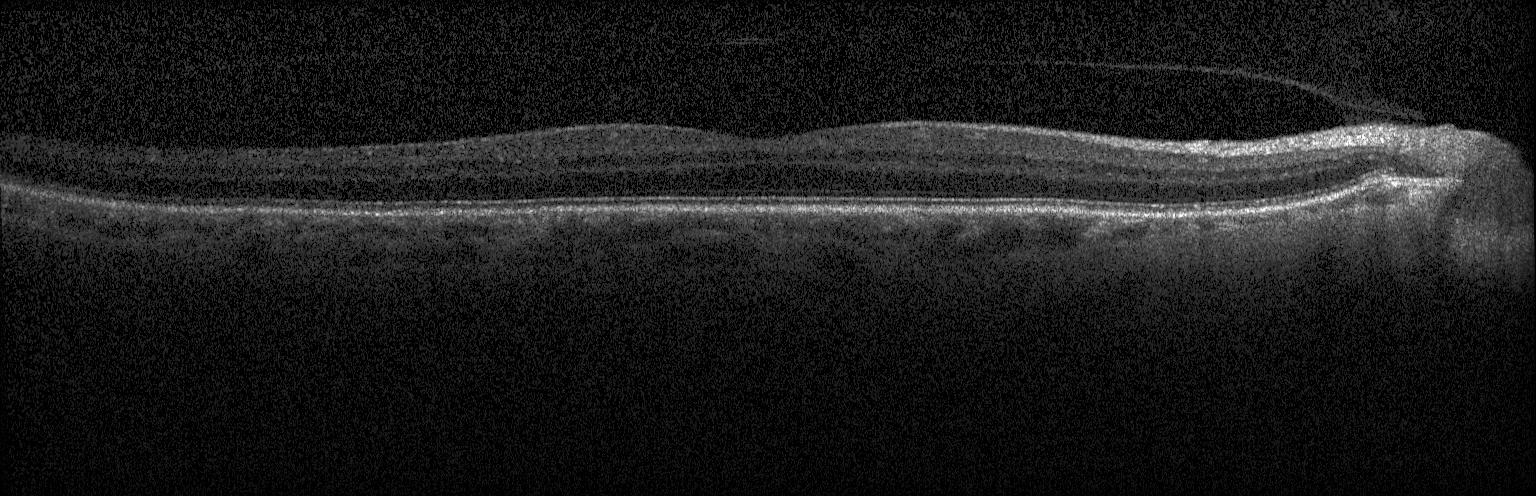
Instrument: Heidelberg Spectralis, optical coherence tomography B-scan. Diagnosis: no evidence of CNV, DME, or drusen.